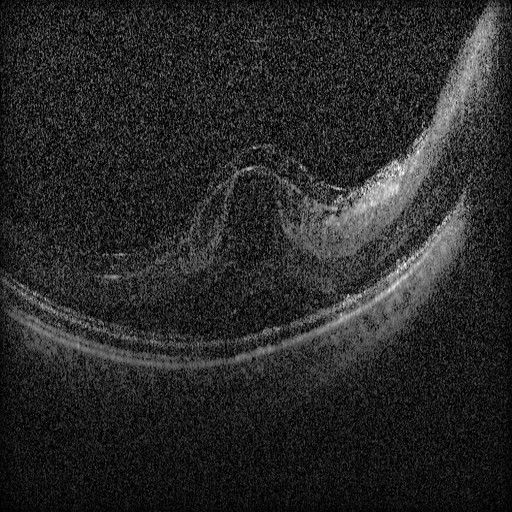
Finding: DME.